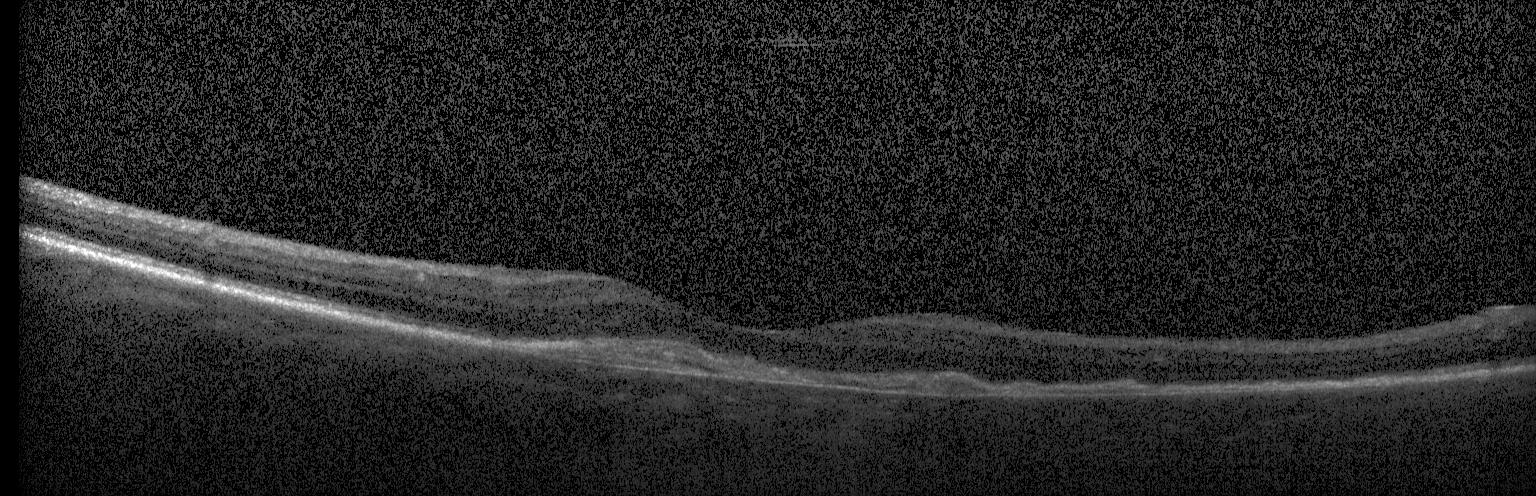
Retinal OCT cross-section · centered on the fovea. Diagnosis: CNV.